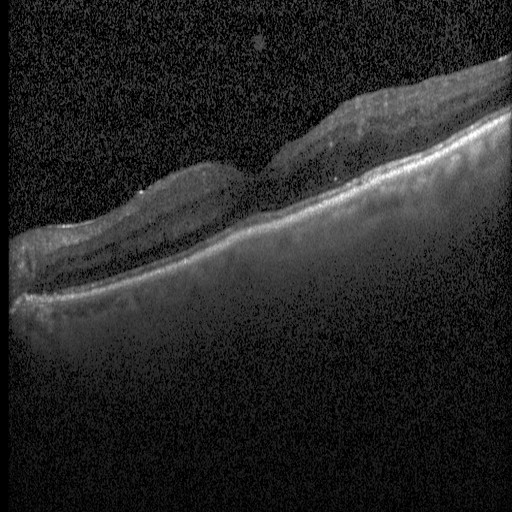 OCT B-scan, macular scan, acquired on a Heidelberg Spectralis.
Diagnosis: DME.